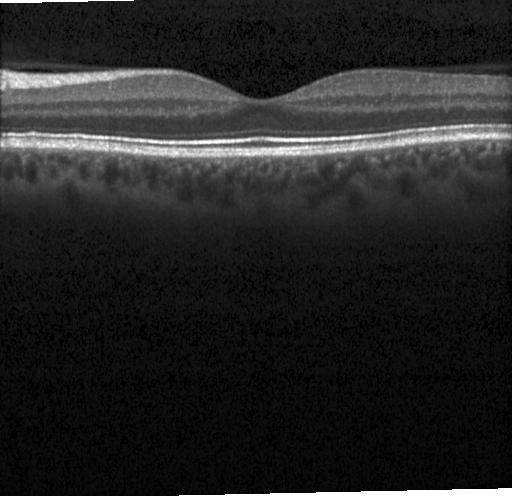
Spectral-domain optical coherence tomography. OCT B-scan. Heidelberg Spectralis OCT system. Macular scan — Impression: no CNV, DME, or drusen.